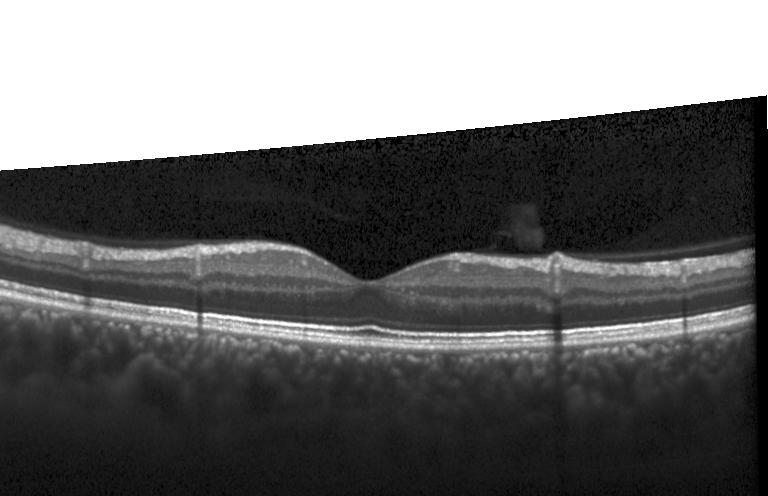

Horizontal scan through the fovea · OCT line scan · instrument: Heidelberg Spectralis · SD-OCT — Diagnosis: neither choroidal neovascularization, diabetic macular edema, nor drusen.